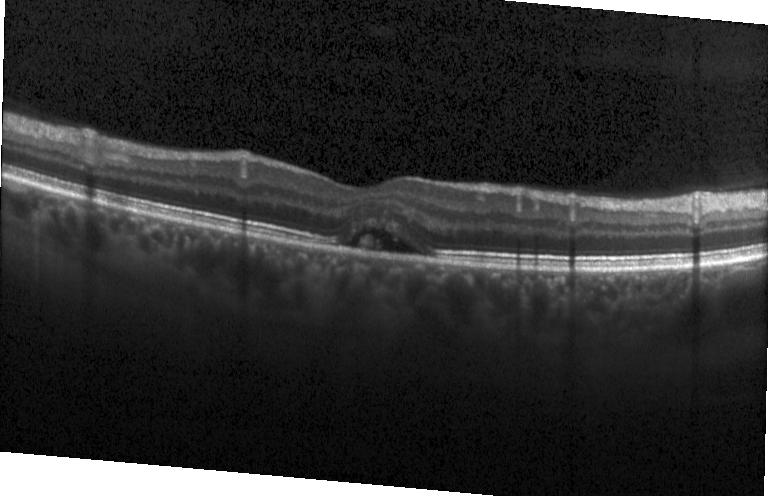 Spectral-domain OCT B-scan: CNV.